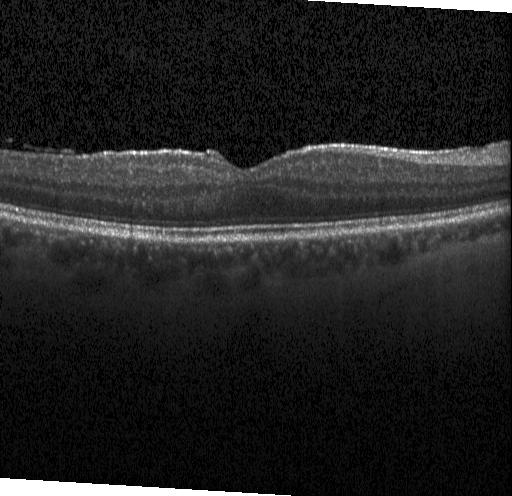

Retinal OCT B-scan; Heidelberg Spectralis OCT system
The scan shows no CNV, no DME, and no drusen.